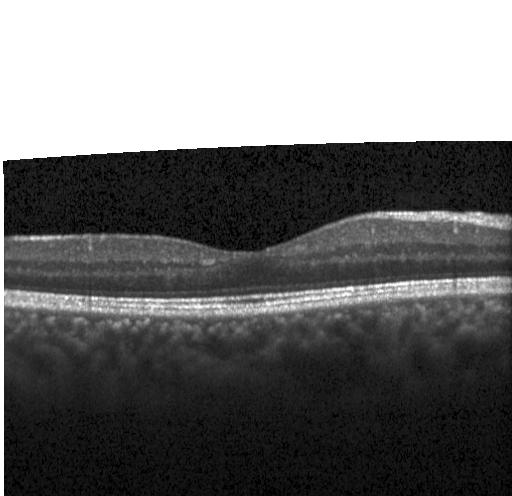 Horizontal scan through the fovea. OCT line scan
Finding: neither CNV, DME, nor drusen.